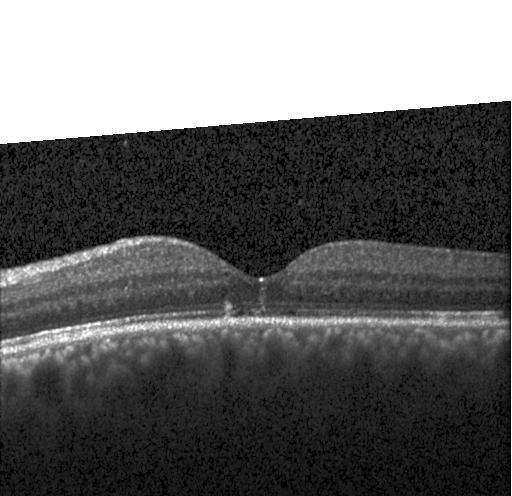

OCT line scan; SD-OCT.
Finding: neither choroidal neovascularization, diabetic macular edema, nor drusen.